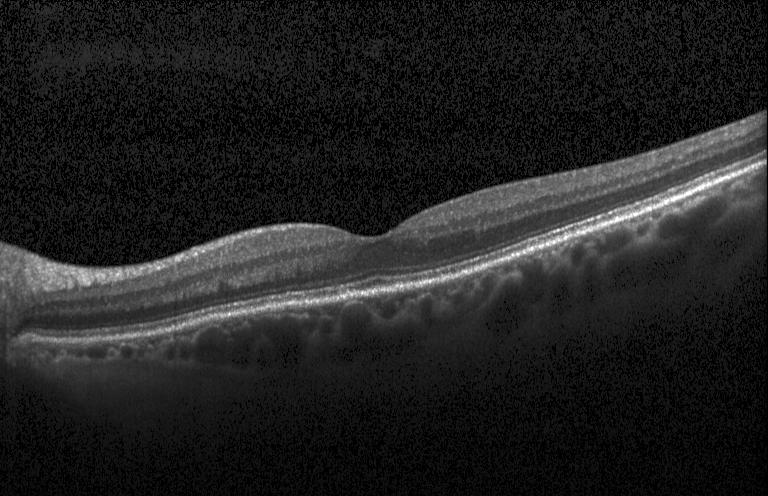
Diagnosis: no choroidal neovascularization, diabetic macular edema, or drusen.